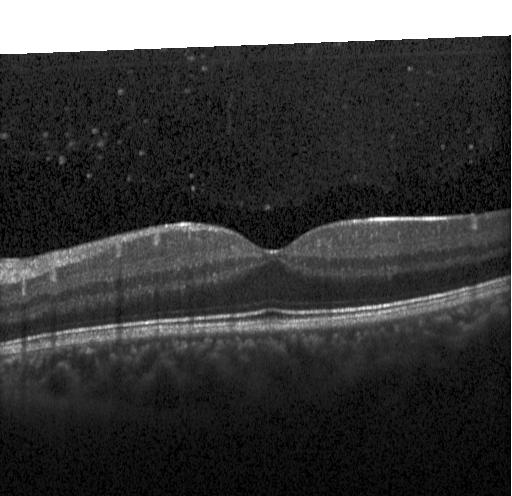 Retinal OCT cross-section showing no evidence of CNV, DME, or drusen.